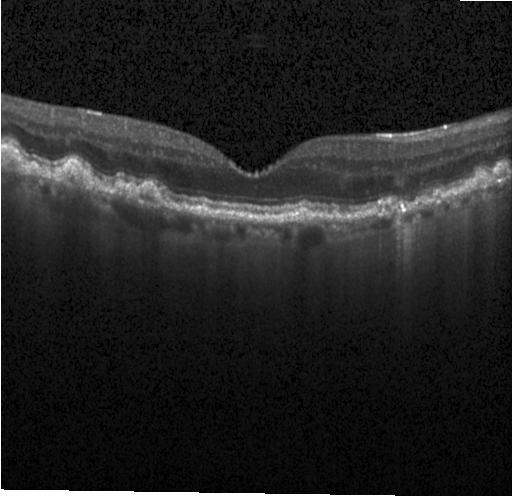 Heidelberg Spectralis · centered on the fovea · optical coherence tomography B-scan — Finding: multiple drusen.